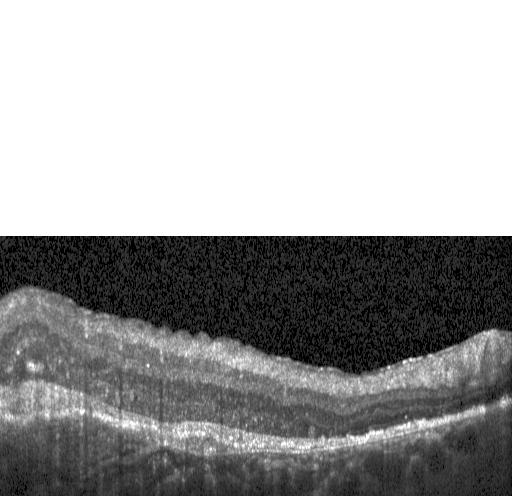 Retinal OCT B-scan · through the macula · Heidelberg Spectralis · spectral-domain optical coherence tomography.
Finding: a choroidal neovascular membrane.